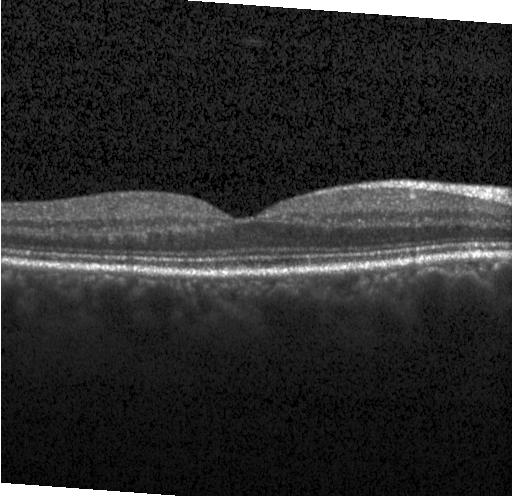 The scan shows no evidence of choroidal neovascularization, diabetic macular edema, or drusen.